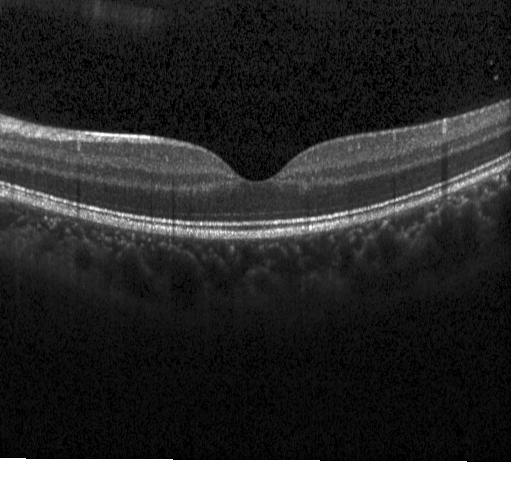 OCT line scan; instrument: Heidelberg Spectralis; centered on the fovea; spectral-domain OCT.
Impression: no choroidal neovascularization, diabetic macular edema, or drusen.